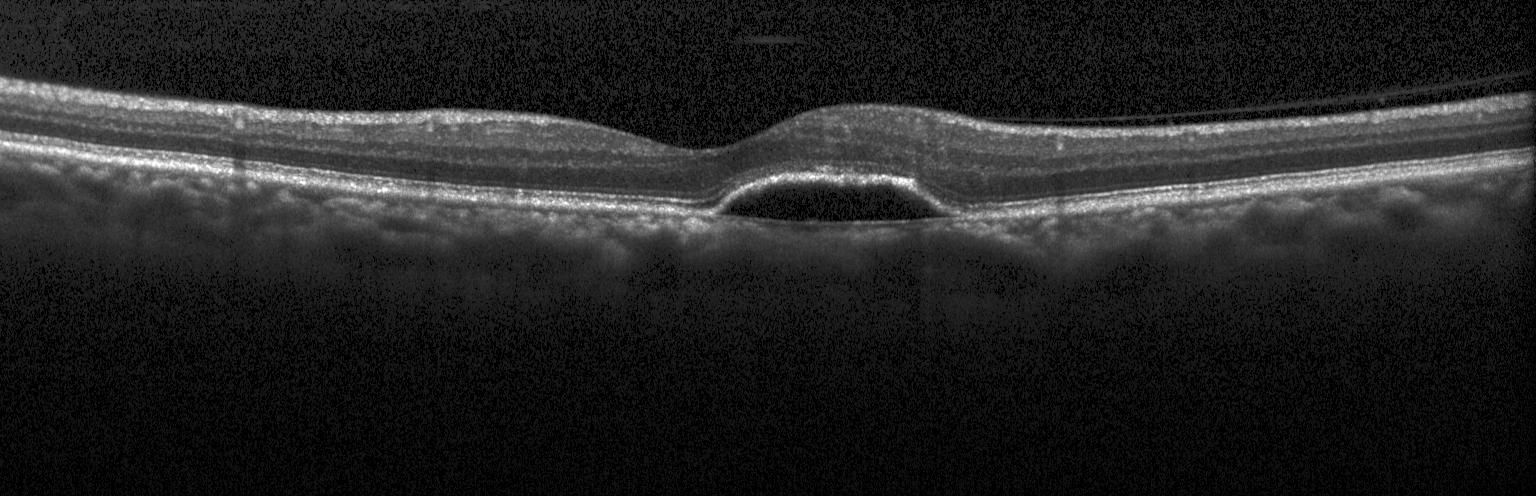
Through the macula. Acquired on a Heidelberg Spectralis. Retinal OCT B-scan. The scan shows a choroidal neovascular membrane.